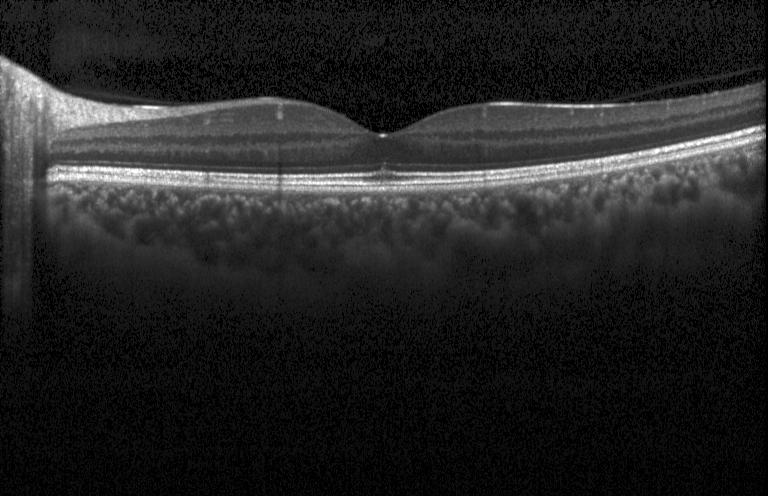
Heidelberg Spectralis, spectral-domain OCT, through the macula, retinal OCT cross-section.
Diagnosis: no choroidal neovascularization, diabetic macular edema, or drusen.